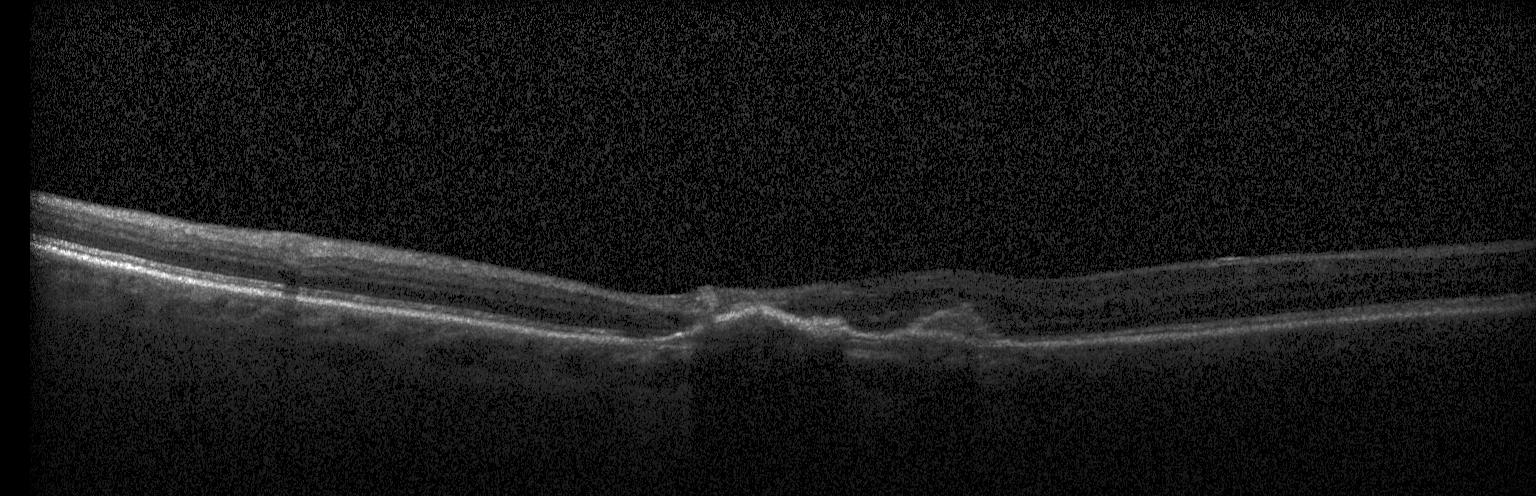 Optical coherence tomography B-scan. SD-OCT. Fovea-centered.
A choroidal neovascular membrane.